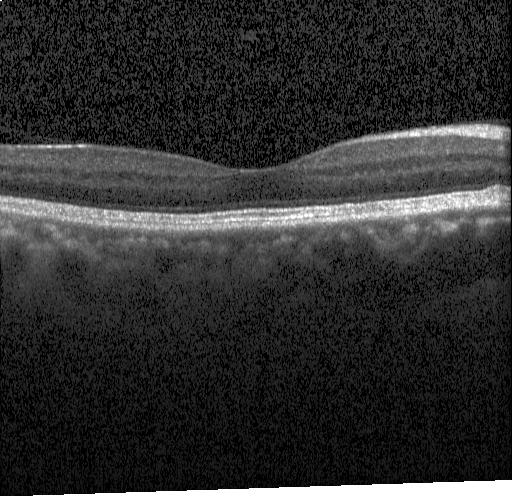

Optical coherence tomography B-scan · acquired on a Heidelberg Spectralis. Macular OCT: neither CNV, DME, nor drusen.